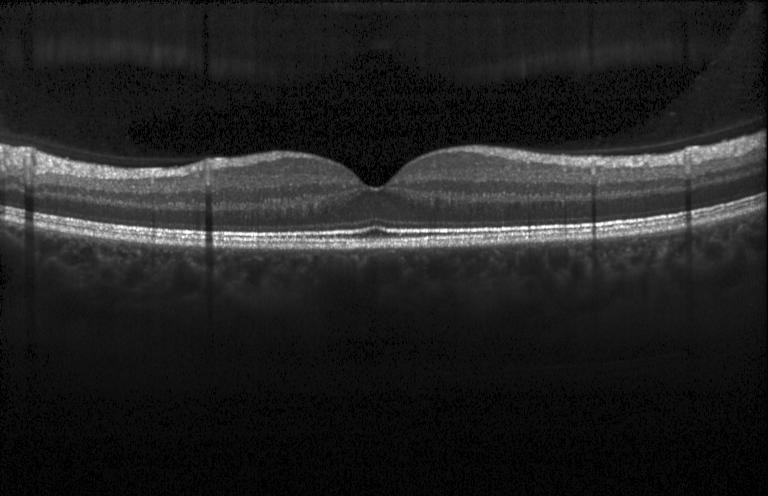
Finding: no choroidal neovascularization, no diabetic macular edema, and no drusen.